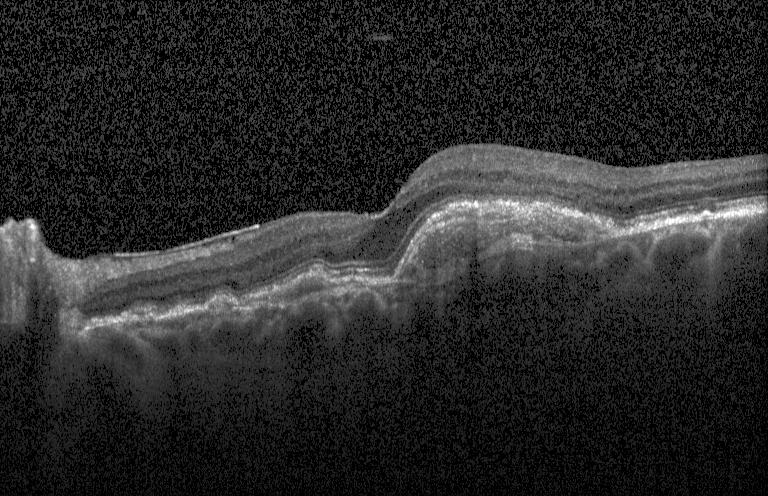 Spectral-domain OCT B-scan: a choroidal neovascular membrane.